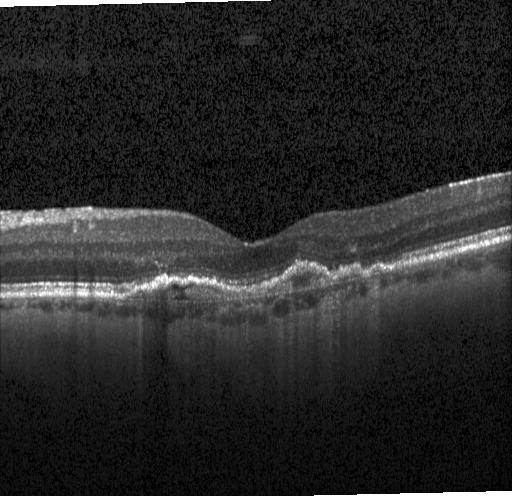
Heidelberg Spectralis OCT system. OCT B-scan. Macular scan — Diagnosis: a choroidal neovascular membrane.